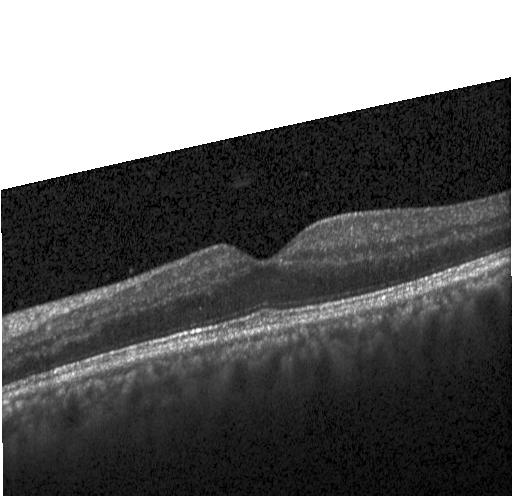

OCT line scan, through the macula.
Impression: no evidence of choroidal neovascularization, diabetic macular edema, or drusen.